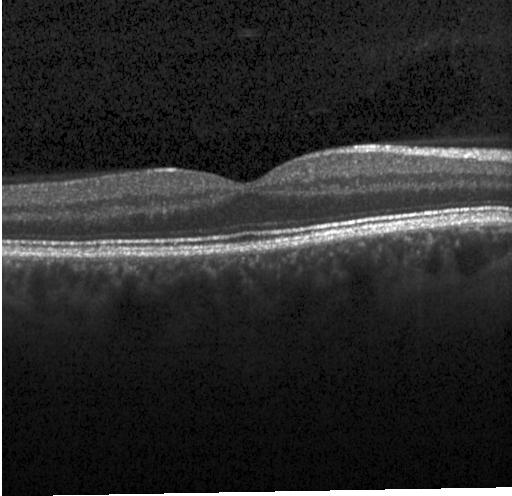

Dx: no CNV, DME, or drusen.